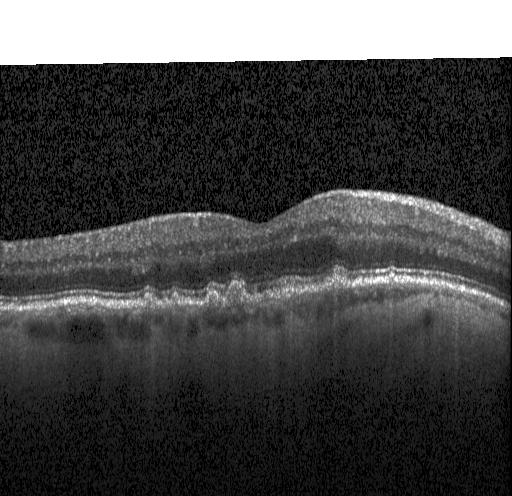 Heidelberg Spectralis OCT system. OCT B-scan — Multiple drusen.